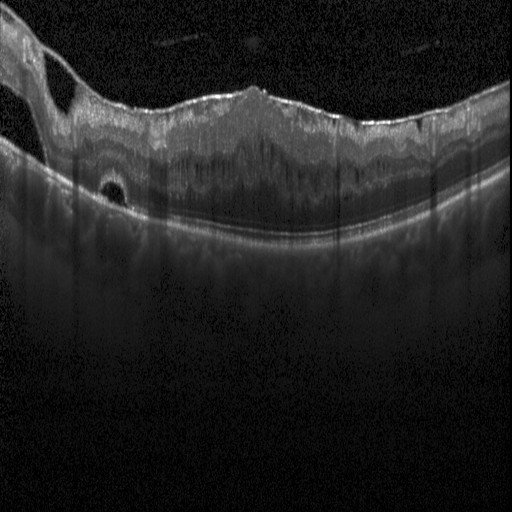 Spectral-domain OCT. OCT line scan. Through the macula
Diabetic macular edema.